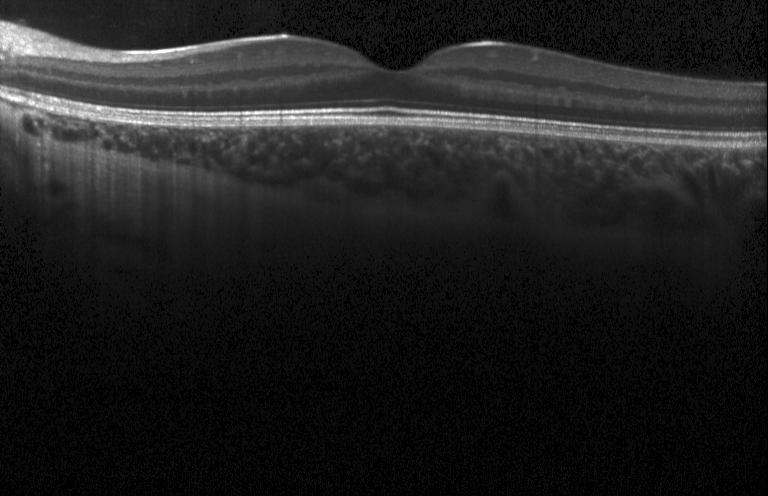
OCT B-scan showing no CNV, DME, or drusen.